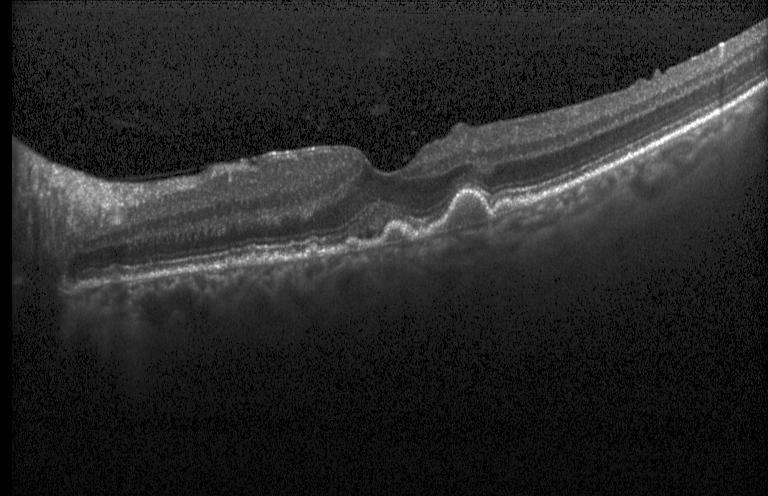
Heidelberg Spectralis; through the macula; retinal OCT B-scan.
Impression: multiple drusen.